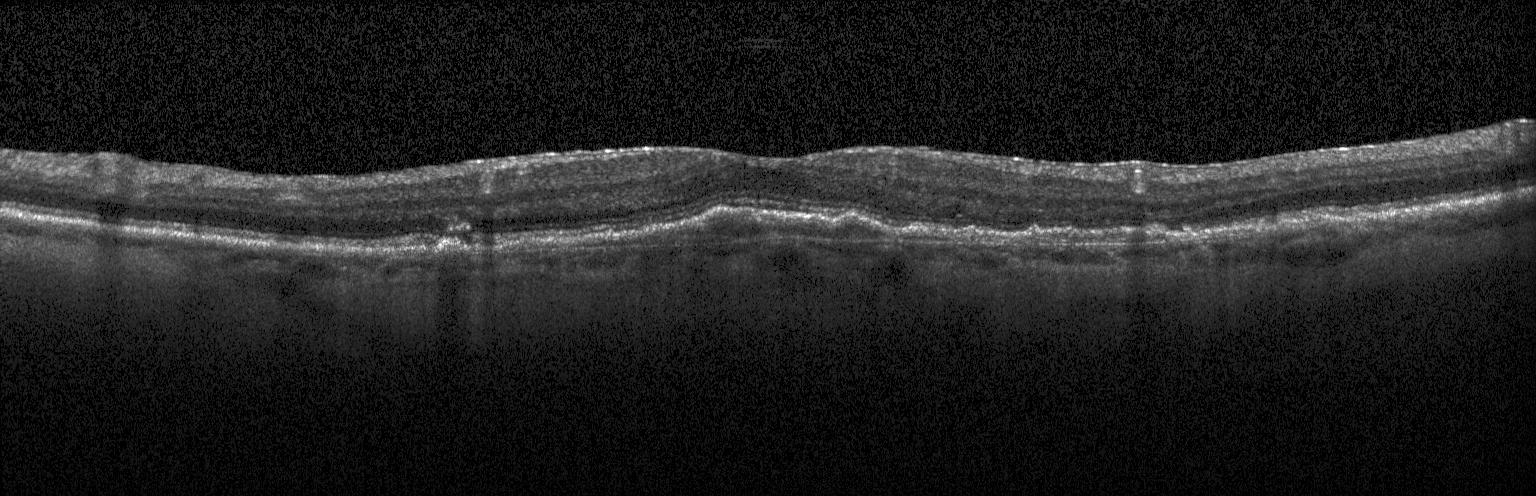

This B-scan demonstrates choroidal neovascularization (CNV).